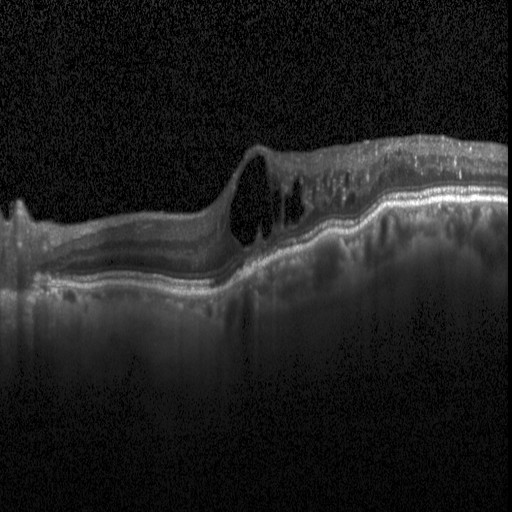

Centered on the fovea, optical coherence tomography scan. Diagnosis: diabetic macular edema.